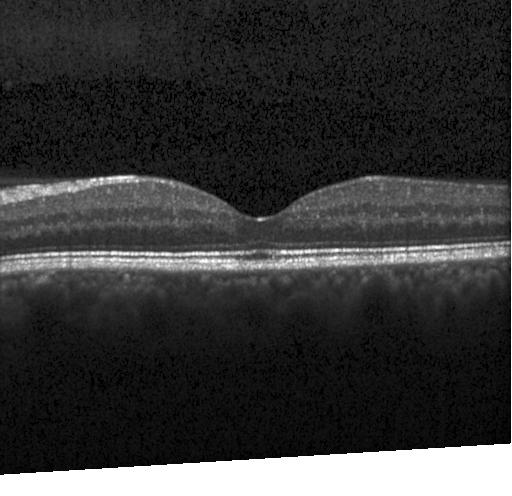

Diagnosis: no choroidal neovascularization, no diabetic macular edema, and no drusen.